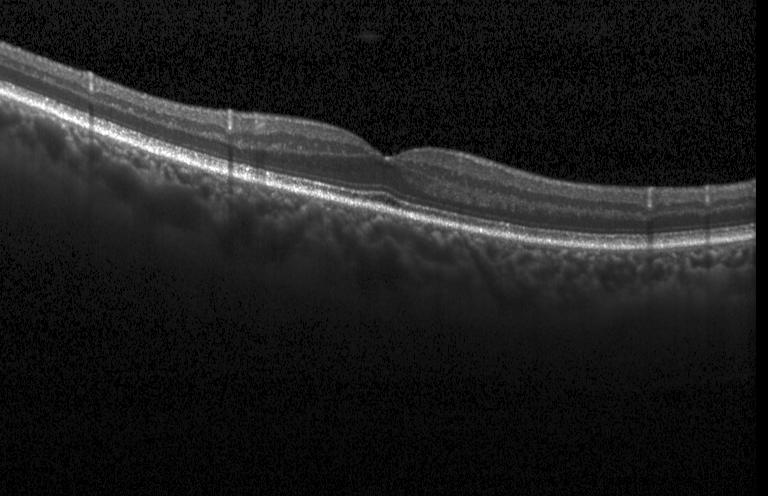

Macular scan; retinal OCT cross-section — OCT finding: no CNV, DME, or drusen.